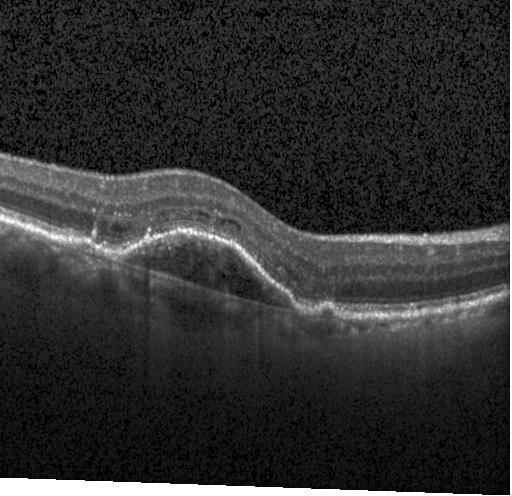

Macular OCT demonstrating choroidal neovascularization (CNV).